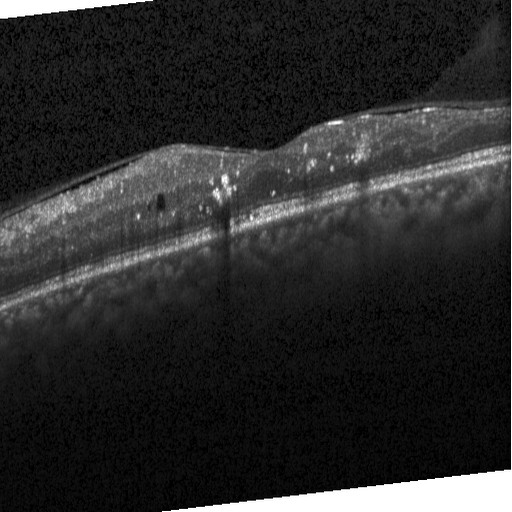
This B-scan demonstrates diabetic macular edema.